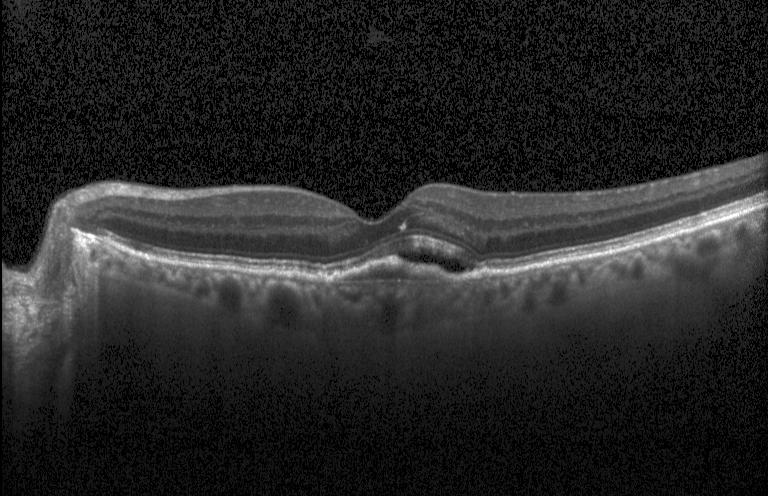 Retinal OCT cross-section
Impression: a choroidal neovascular membrane.